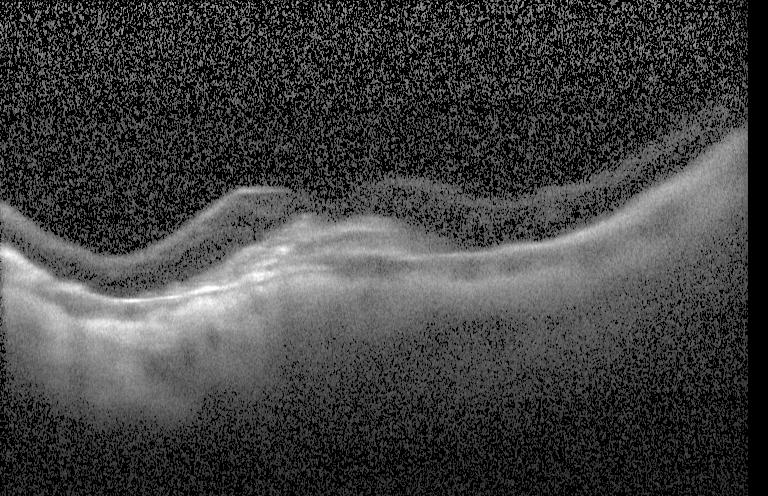

Dx: a choroidal neovascular membrane.